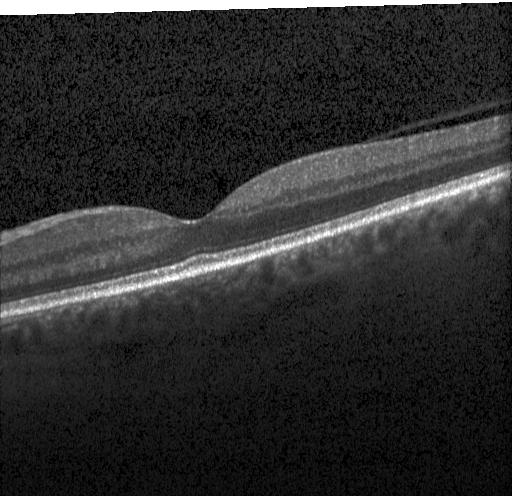 Retinal OCT cross-section showing neither choroidal neovascularization, diabetic macular edema, nor drusen.